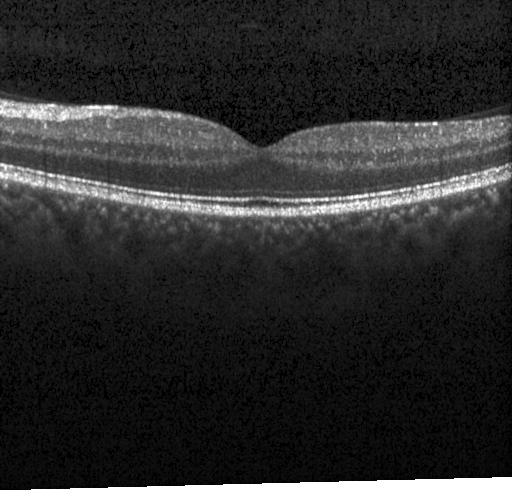

Optical coherence tomography scan; instrument: Heidelberg Spectralis; spectral-domain OCT
Diagnosis: no choroidal neovascularization, diabetic macular edema, or drusen.